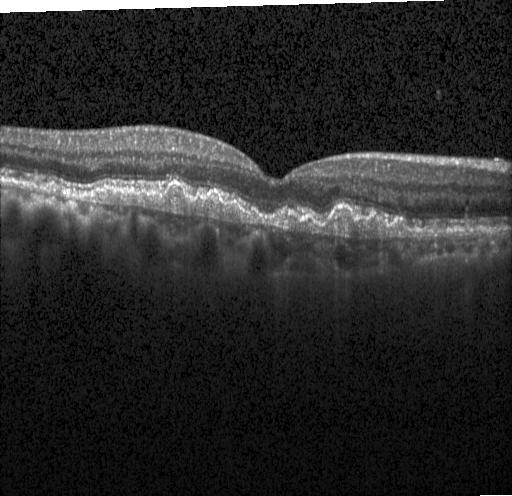 Centered on the fovea · Heidelberg Spectralis OCT system · optical coherence tomography scan · SD-OCT
The scan shows a choroidal neovascular membrane.